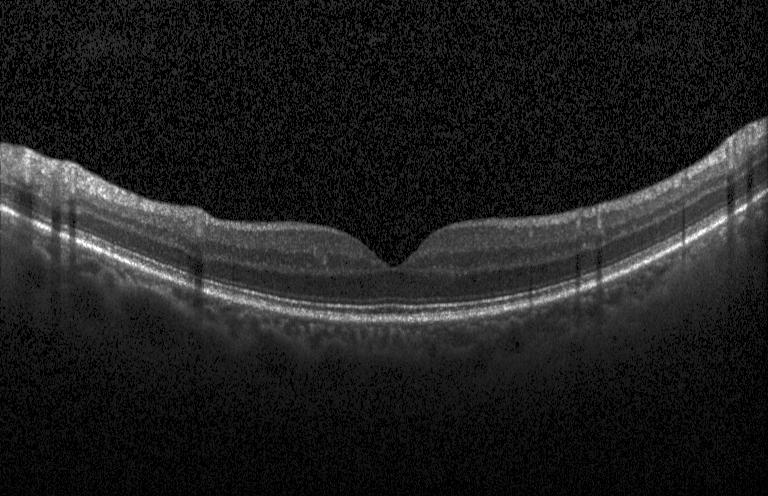 OCT finding: no choroidal neovascularization, no diabetic macular edema, and no drusen.